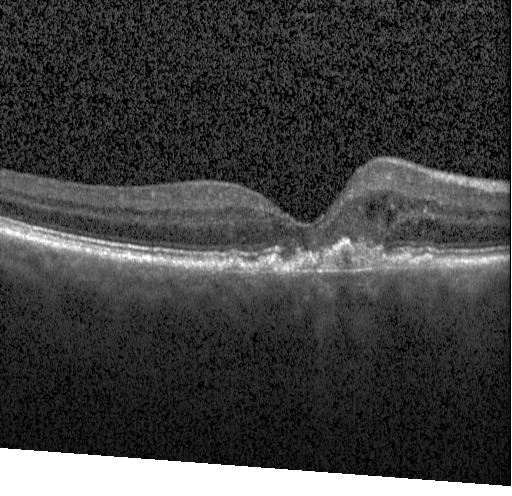 Retinal OCT cross-section showing a choroidal neovascular membrane.